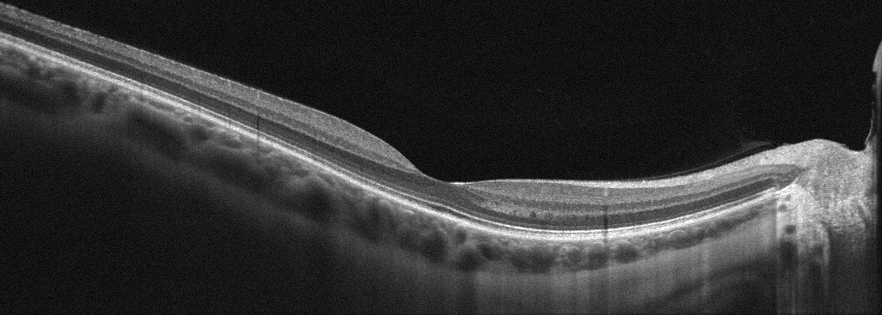

OCT line scan, right eye, through the macula — Macular OCT: absence of AMD, DME, ERM, RAO, RVO, and vitreomacular interface disease.